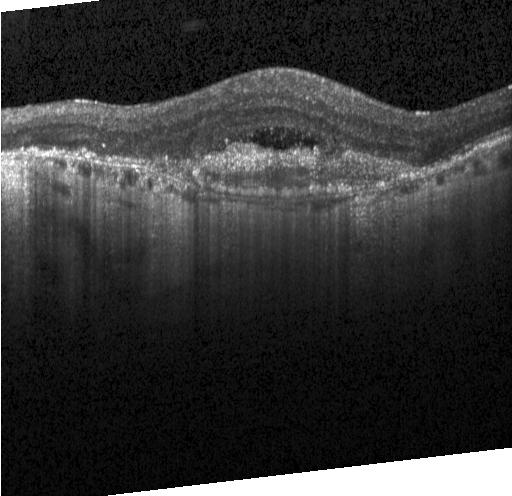

Diagnosis: CNV.